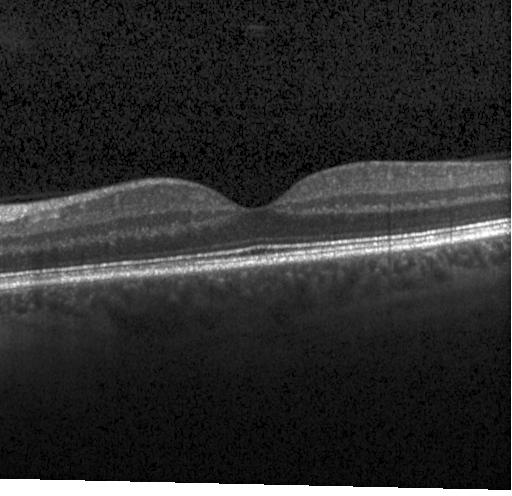

Finding: no evidence of choroidal neovascularization, diabetic macular edema, or drusen.